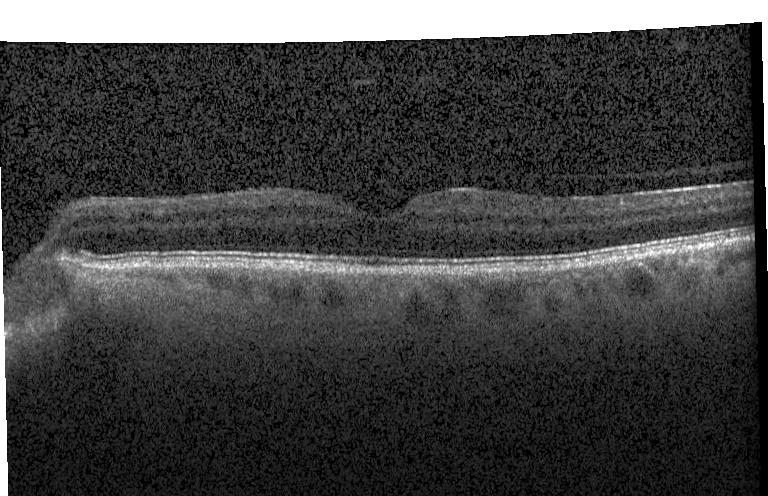
OCT finding: no choroidal neovascularization, no diabetic macular edema, and no drusen.